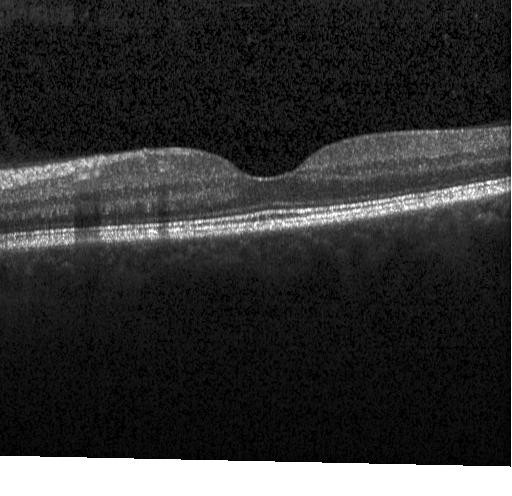
Heidelberg Spectralis OCT system, optical coherence tomography scan — Finding: no CNV, DME, or drusen.